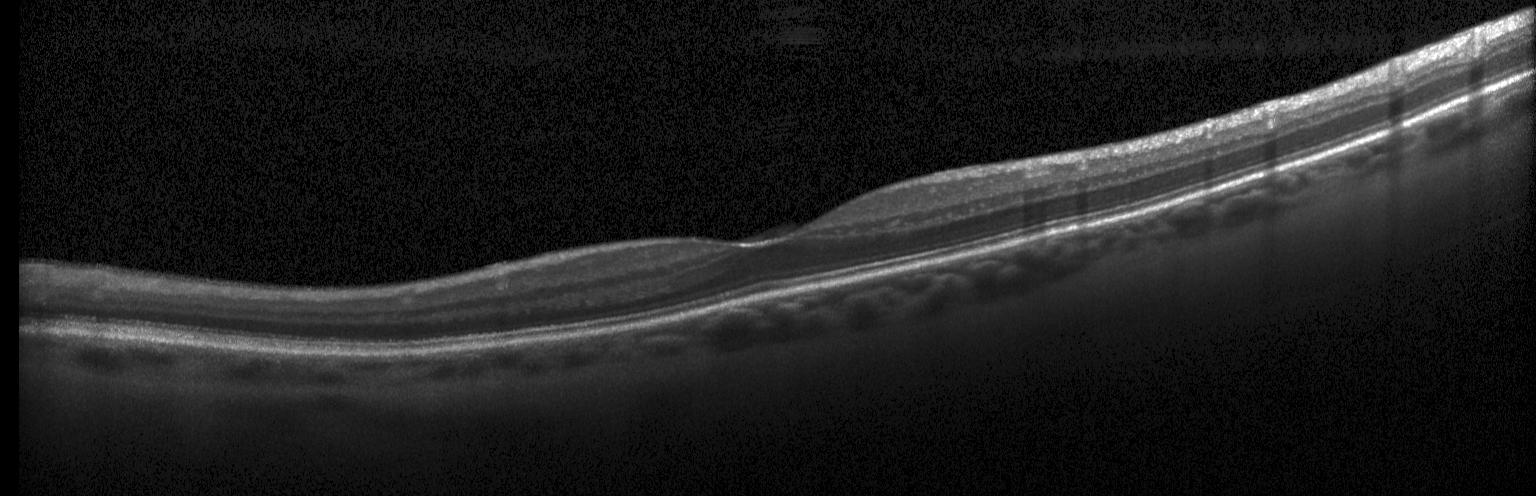

OCT B-scan · SD-OCT — Diagnosis: neither choroidal neovascularization, diabetic macular edema, nor drusen.